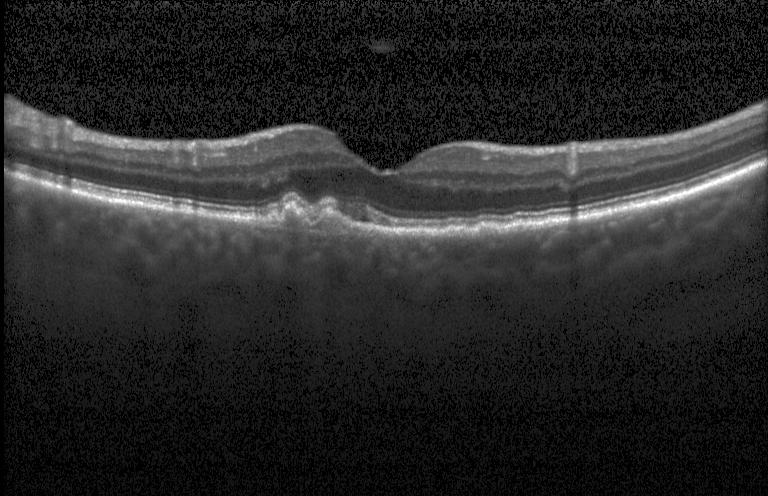
Finding: a choroidal neovascular membrane.